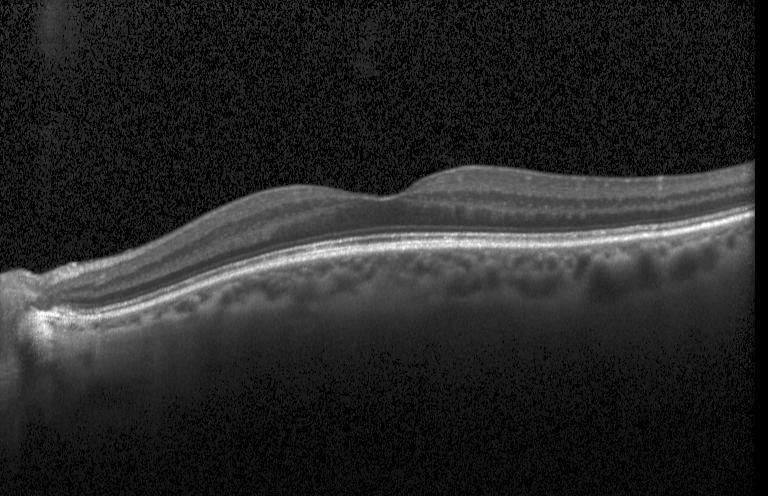 Through the macula, retinal OCT cross-section — No choroidal neovascularization, diabetic macular edema, or drusen.